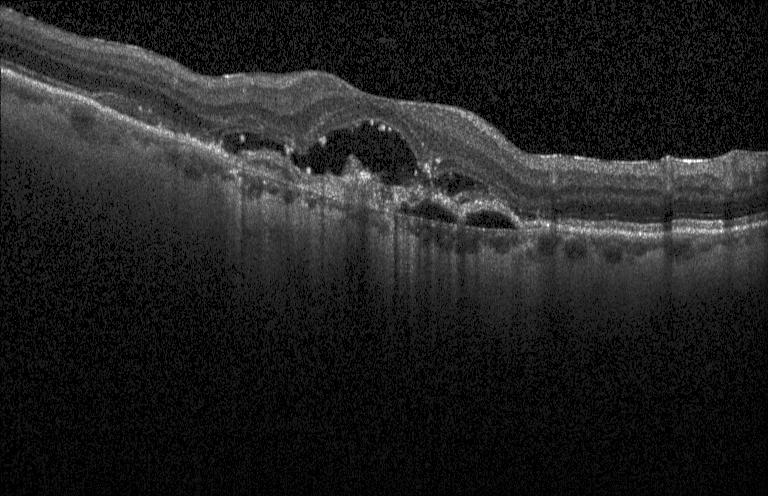

Fovea-centered; spectral-domain optical coherence tomography; Heidelberg Spectralis; retinal OCT cross-section — Finding: CNV.